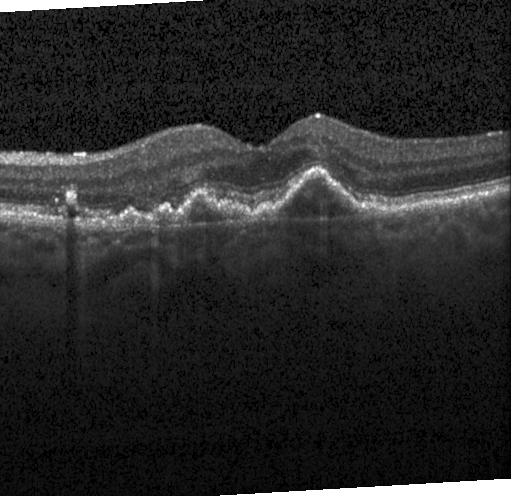

Optical coherence tomography B-scan, fovea-centered, spectral-domain optical coherence tomography, Heidelberg Spectralis — A choroidal neovascular membrane.